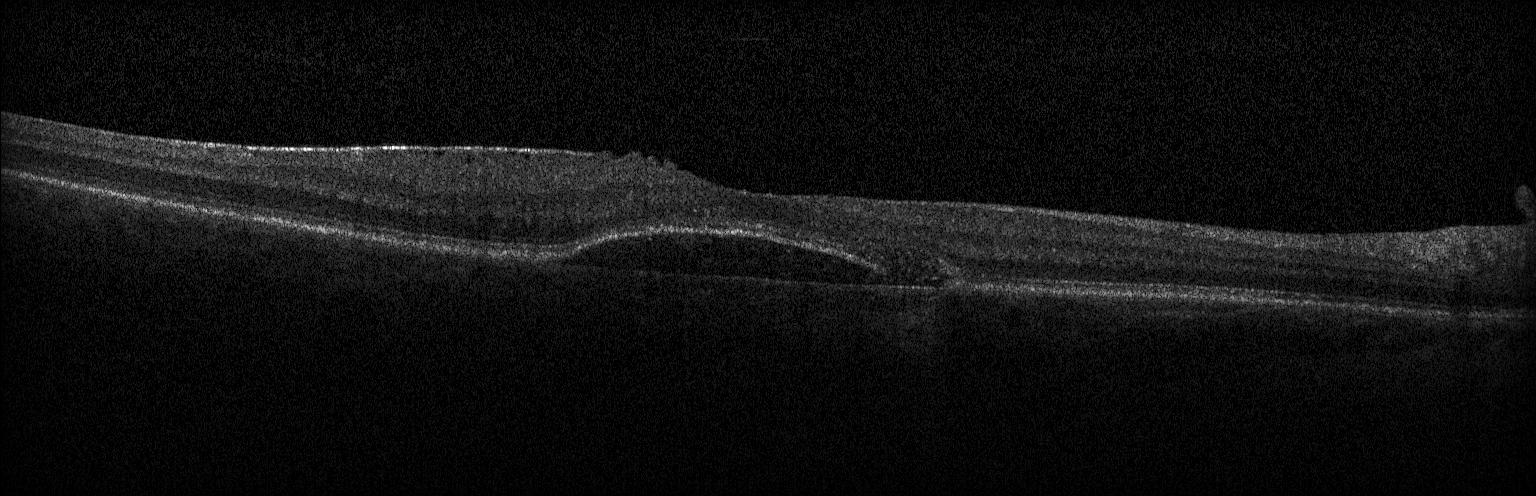
Heidelberg Spectralis. OCT B-scan. Spectral-domain optical coherence tomography — OCT finding: a choroidal neovascular membrane.